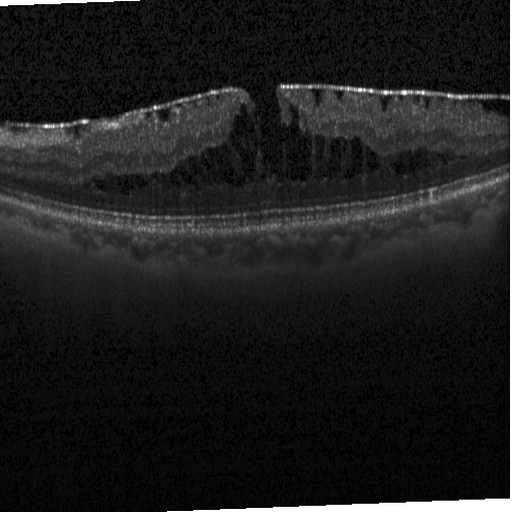 Instrument: Heidelberg Spectralis, through the macula, spectral-domain optical coherence tomography, optical coherence tomography B-scan
Diagnosis: DME.